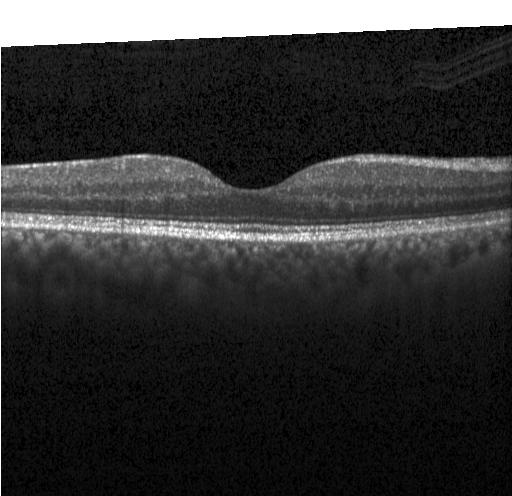

Fovea-centered · optical coherence tomography B-scan · Heidelberg Spectralis
This B-scan demonstrates no evidence of CNV, DME, or drusen.